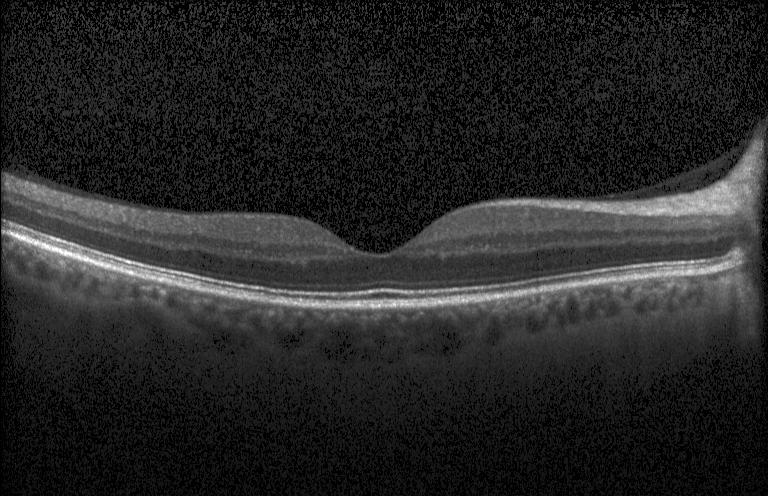 Finding: no choroidal neovascularization, diabetic macular edema, or drusen.